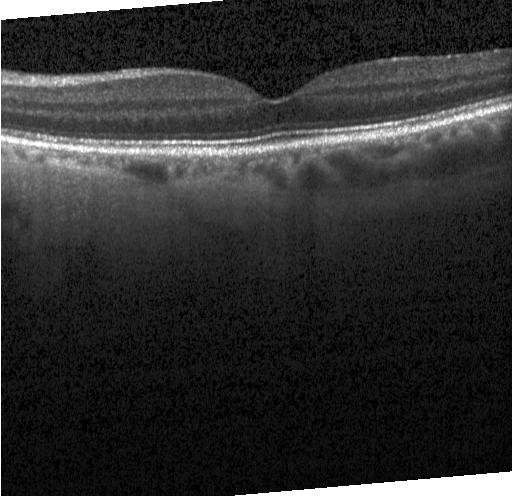

Assessment: no evidence of choroidal neovascularization, diabetic macular edema, or drusen.